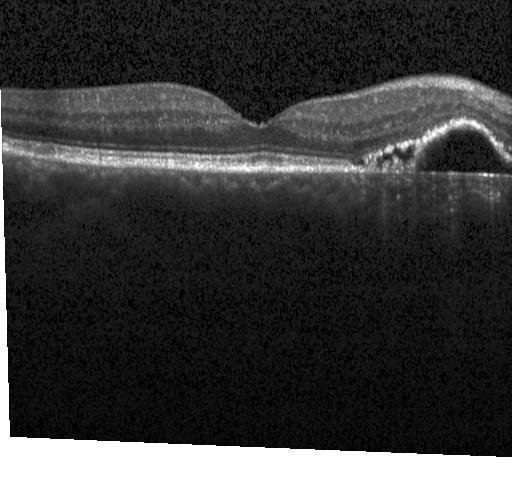

Retinal OCT cross-section, horizontal scan through the fovea.
Assessment: CNV.